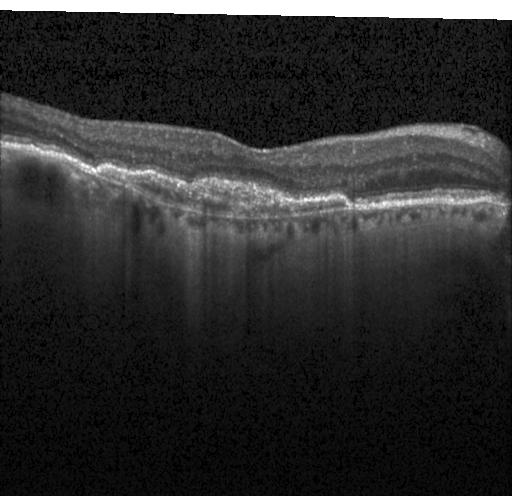

Heidelberg Spectralis. Optical coherence tomography scan
A choroidal neovascular membrane.